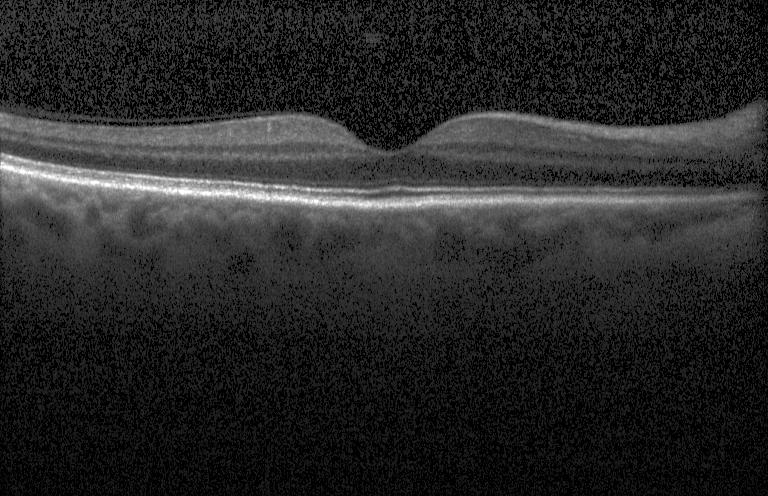
Retinal OCT B-scan.
Assessment: no CNV, no DME, and no drusen.